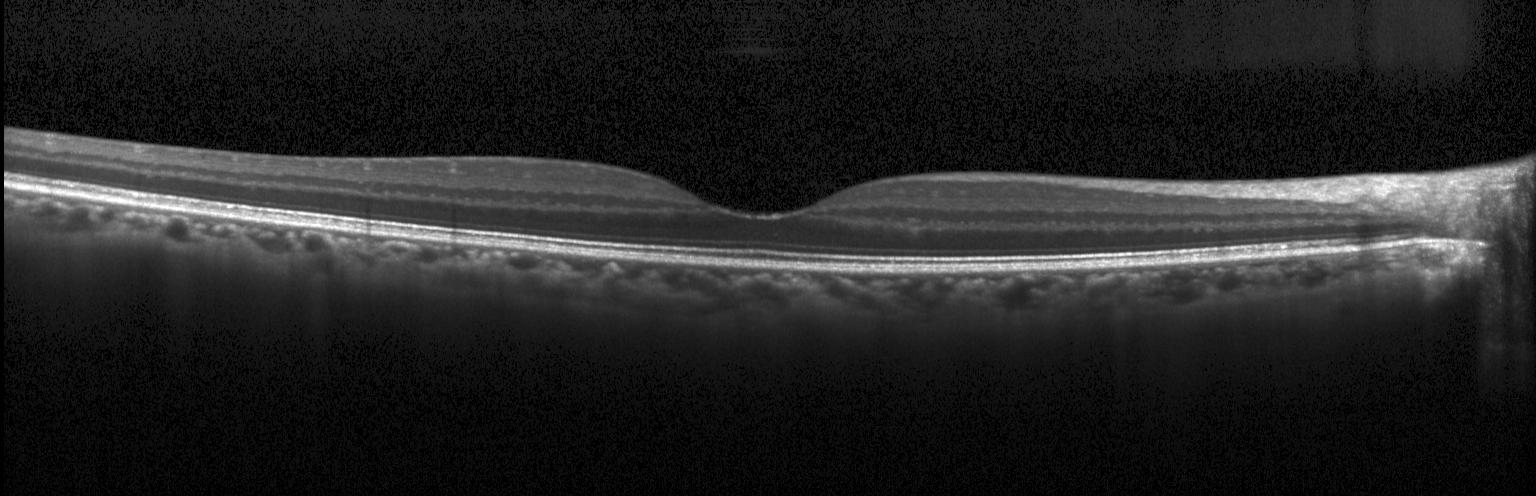

Retinal OCT B-scan
OCT finding: no choroidal neovascularization, diabetic macular edema, or drusen.